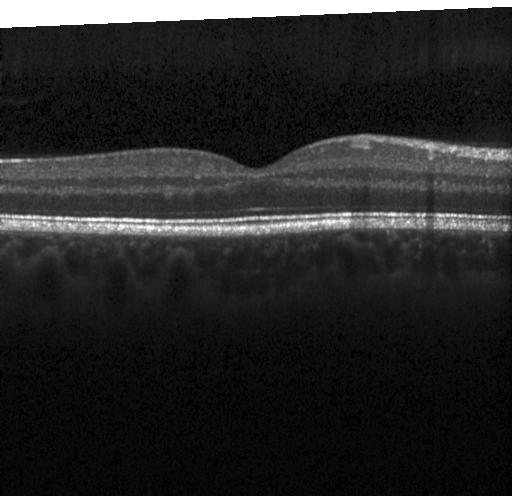 Optical coherence tomography B-scan · acquired on a Heidelberg Spectralis · spectral-domain optical coherence tomography · centered on the fovea — Finding: neither choroidal neovascularization, diabetic macular edema, nor drusen.